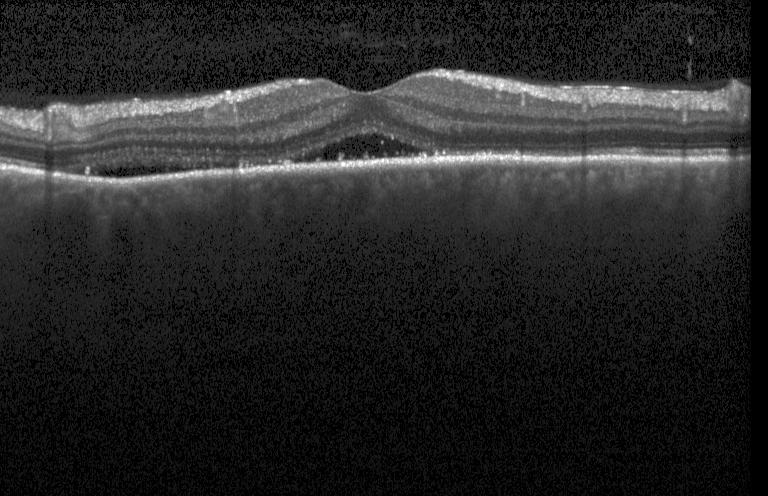

Impression: choroidal neovascularization (CNV).